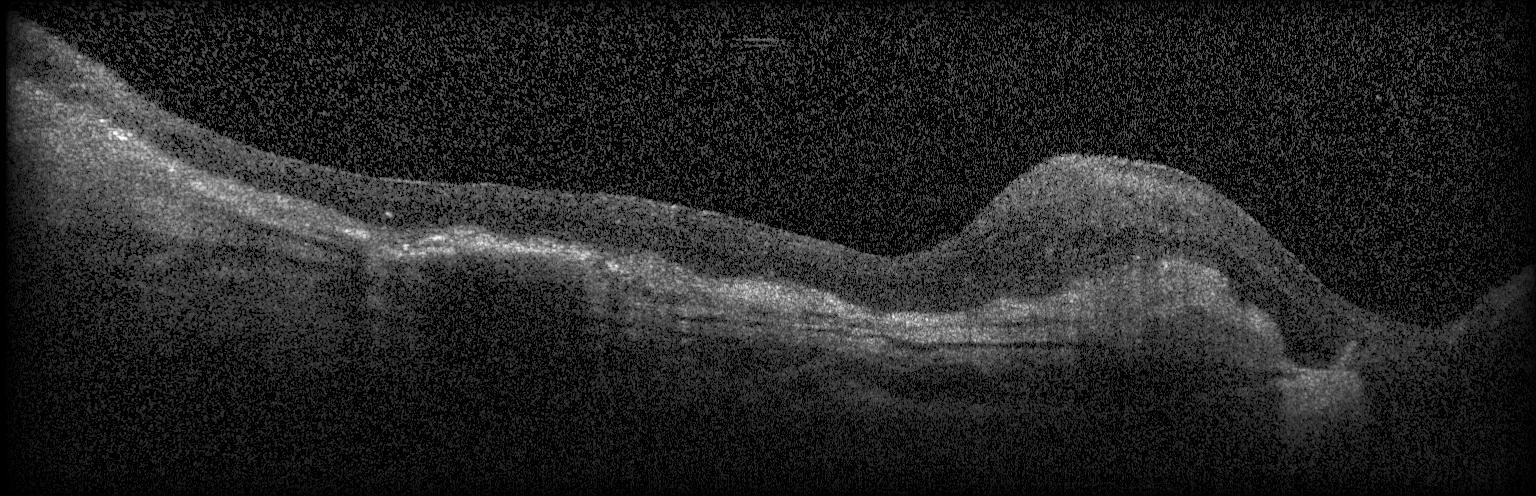
Retinal OCT cross-section. Horizontal scan through the fovea. Acquired on a Heidelberg Spectralis. Spectral-domain optical coherence tomography
OCT finding: CNV.